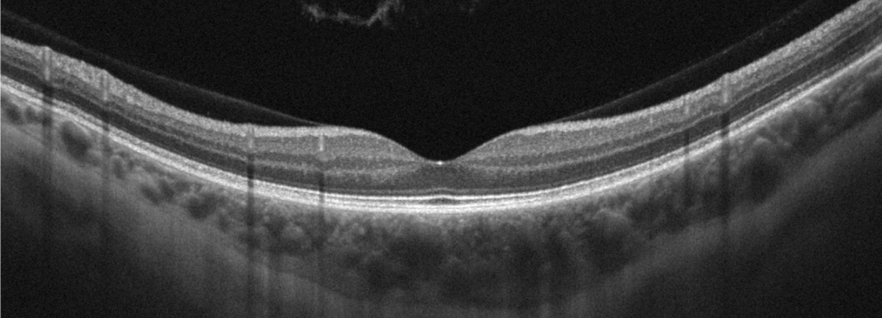 Through the macula · retinal OCT cross-section — Absence of AMD, DME, ERM, RAO, RVO, and vitreomacular interface disease.